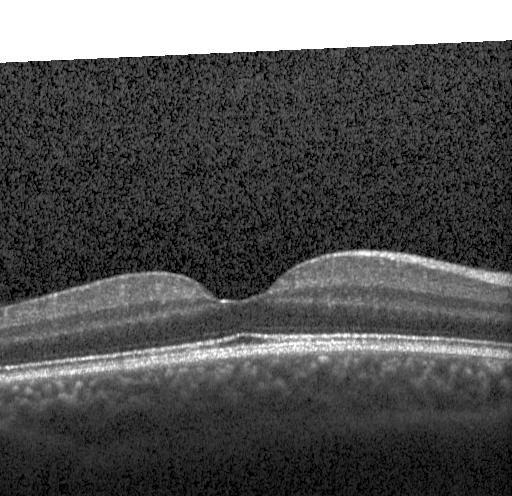

Diagnosis: no CNV, DME, or drusen.